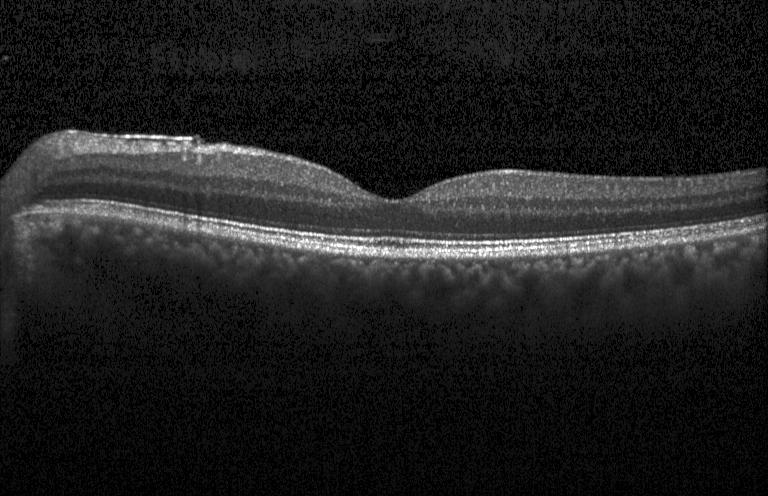 Instrument: Heidelberg Spectralis, SD-OCT, OCT B-scan — Impression: neither choroidal neovascularization, diabetic macular edema, nor drusen.